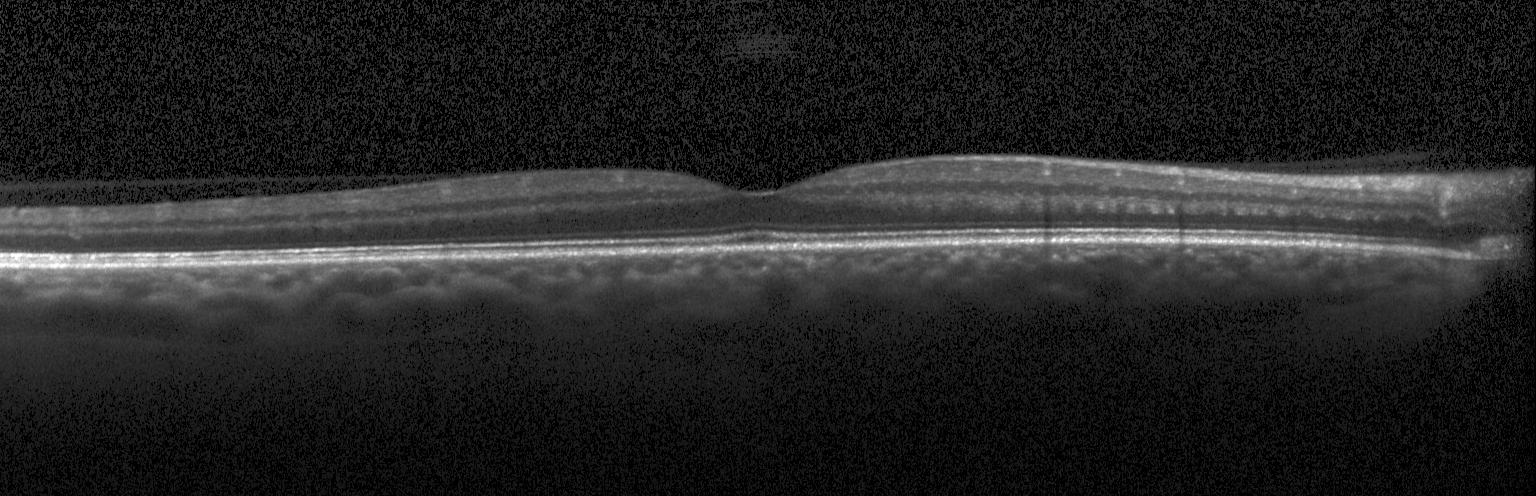 Impression: no evidence of CNV, DME, or drusen.